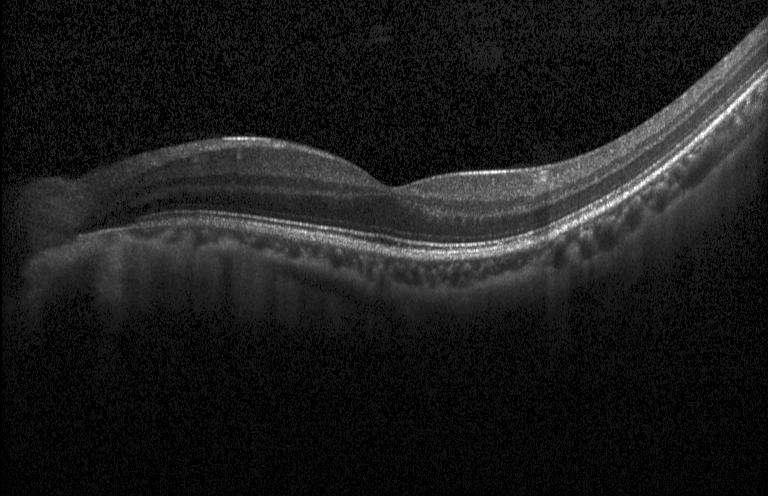
Spectral-domain optical coherence tomography. Optical coherence tomography scan
Impression: no evidence of choroidal neovascularization, diabetic macular edema, or drusen.